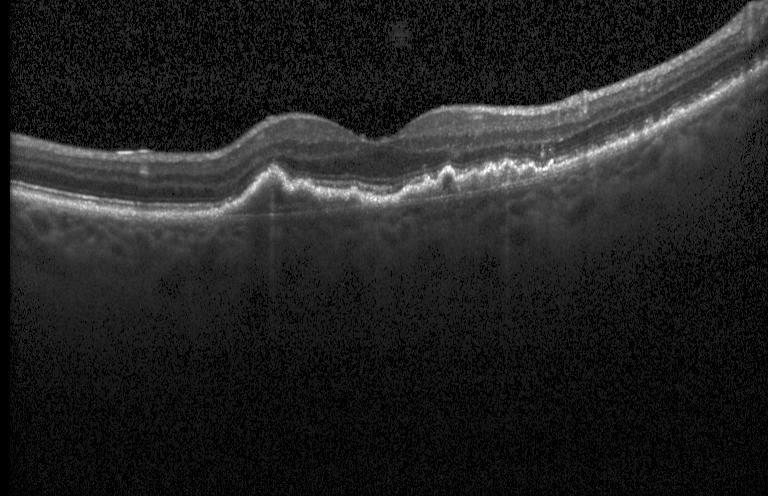
OCT B-scan. Through the macula. Spectral-domain OCT. This B-scan demonstrates a choroidal neovascular membrane.